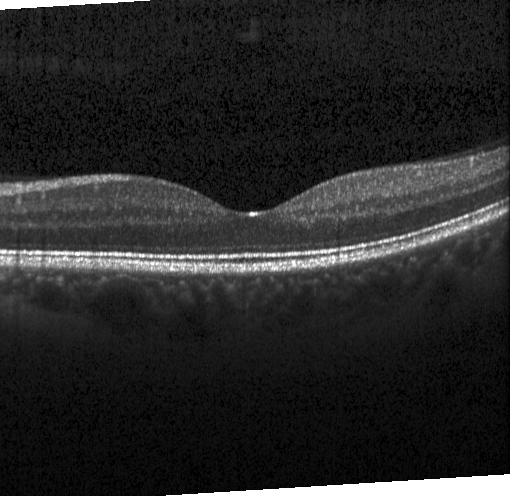
OCT line scan — This B-scan demonstrates no choroidal neovascularization, no diabetic macular edema, and no drusen.